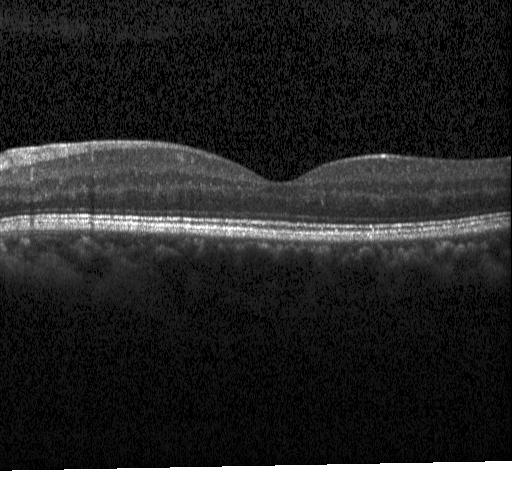
Heidelberg Spectralis OCT system · optical coherence tomography scan · spectral-domain OCT.
Diagnosis: no evidence of choroidal neovascularization, diabetic macular edema, or drusen.